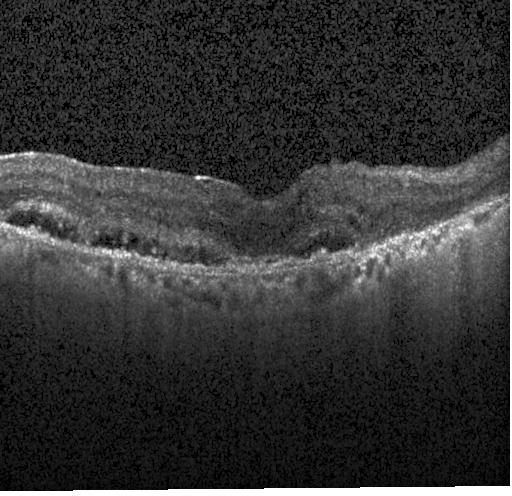

Heidelberg Spectralis. Optical coherence tomography scan. Fovea-centered
Dx: a choroidal neovascular membrane.